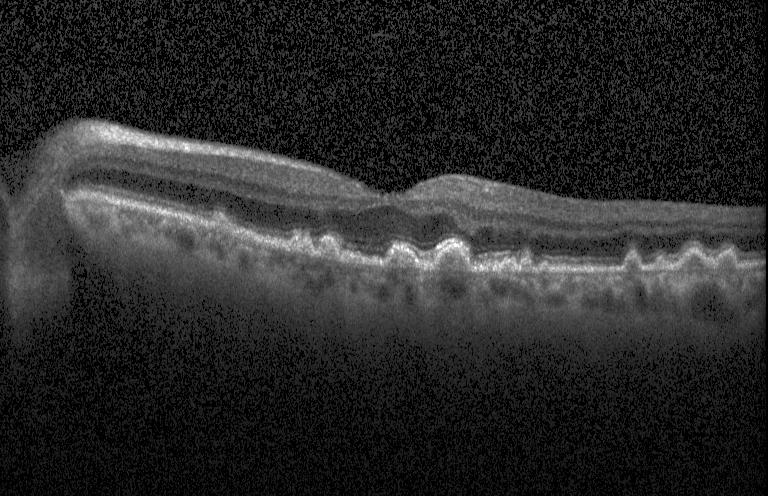

Diagnosis: sub-RPE drusenoid deposits.